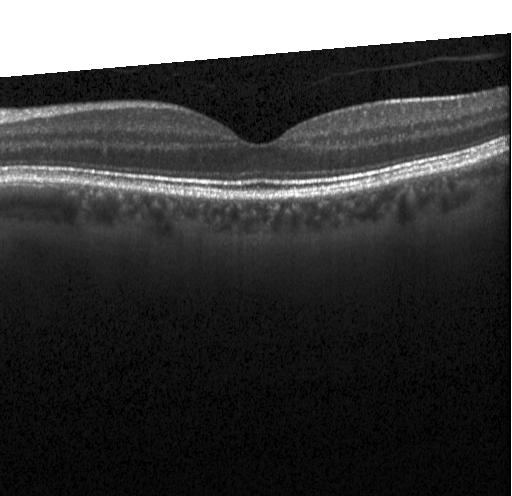 Impression: no choroidal neovascularization, diabetic macular edema, or drusen.